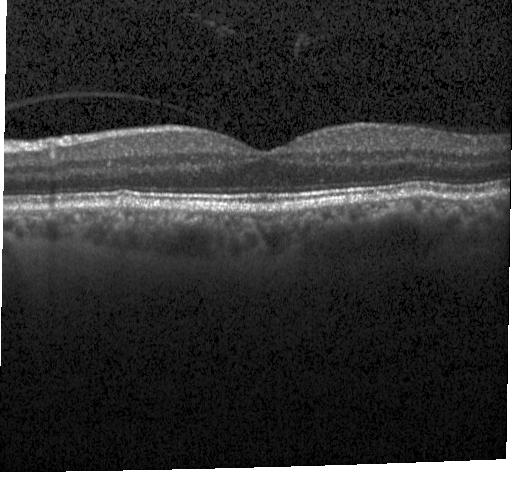 OCT B-scan showing no choroidal neovascularization, diabetic macular edema, or drusen.